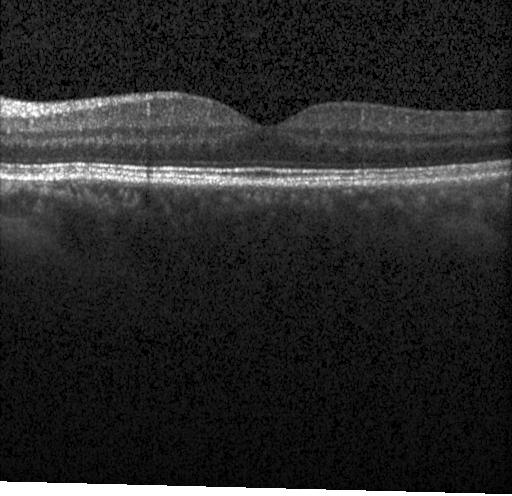
Retinal OCT cross-section; Heidelberg Spectralis; spectral-domain OCT. The scan shows no choroidal neovascularization, no diabetic macular edema, and no drusen.